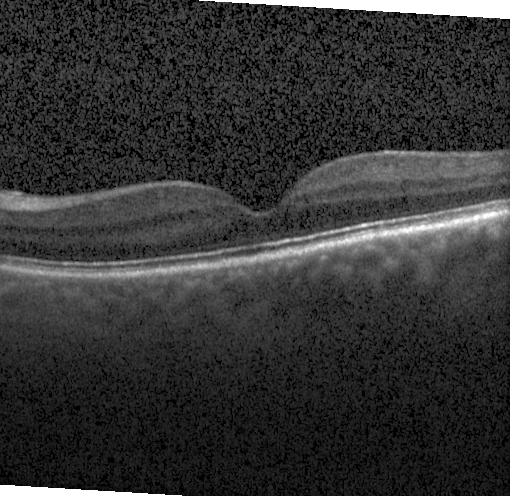

Optical coherence tomography B-scan
This B-scan demonstrates neither choroidal neovascularization, diabetic macular edema, nor drusen.